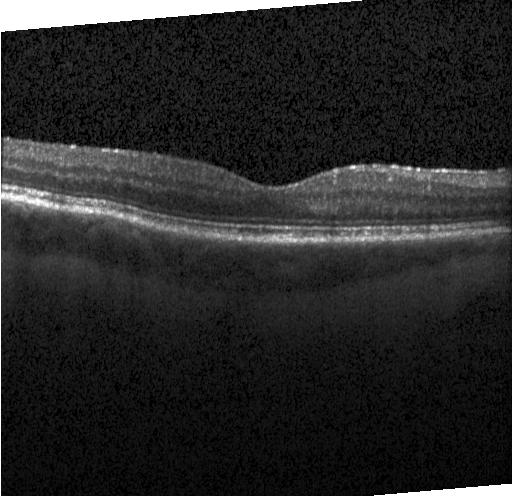

Impression: no CNV, DME, or drusen.